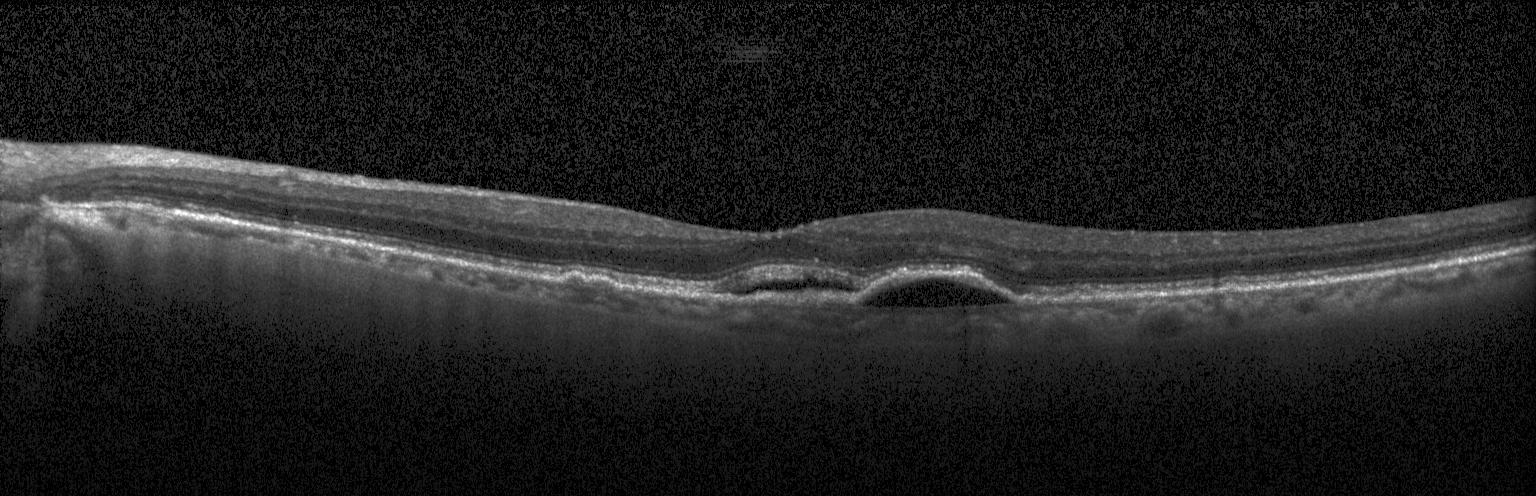 OCT scan showing choroidal neovascularization (CNV).